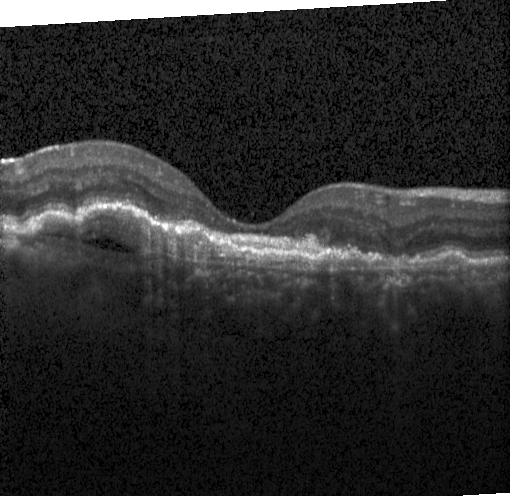 OCT line scan. Acquired on a Heidelberg Spectralis. Centered on the fovea. Spectral-domain OCT — Macular OCT: CNV.